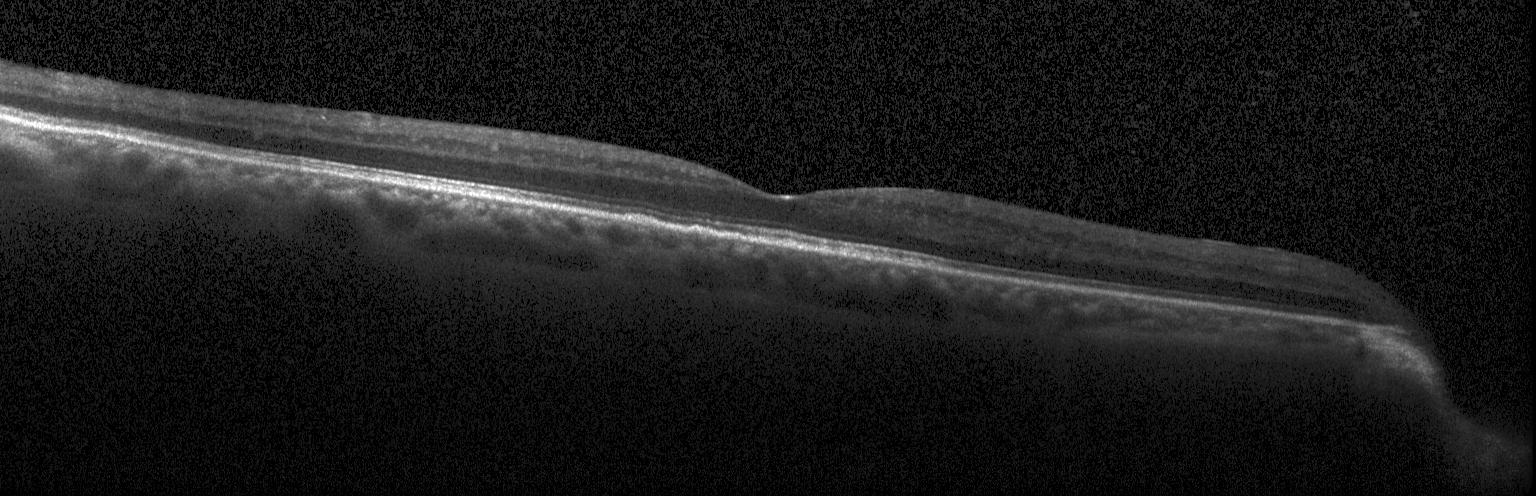
Optical coherence tomography scan; spectral-domain optical coherence tomography. Finding: neither CNV, DME, nor drusen.